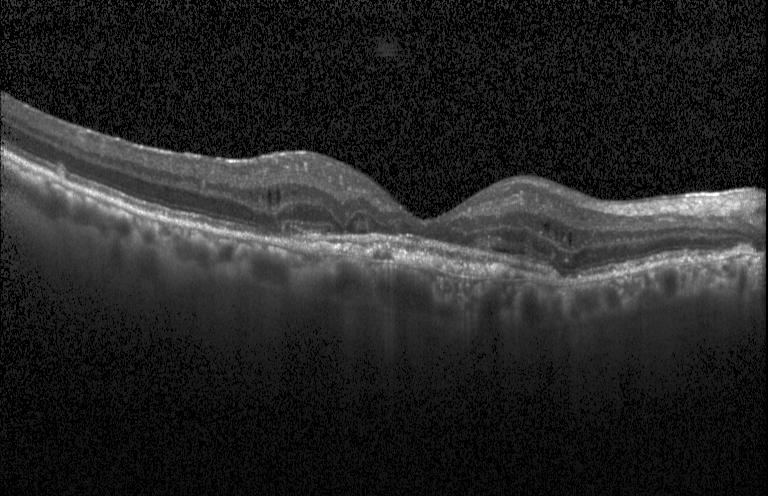 Retinal OCT cross-section, spectral-domain OCT
Diagnosis: a choroidal neovascular membrane.